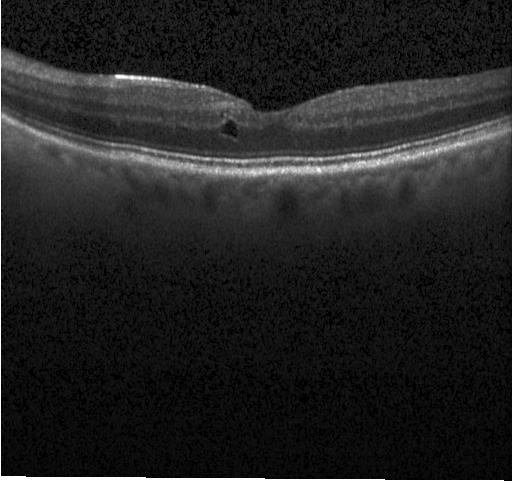 Optical coherence tomography scan. Impression: diabetic macular edema (DME).